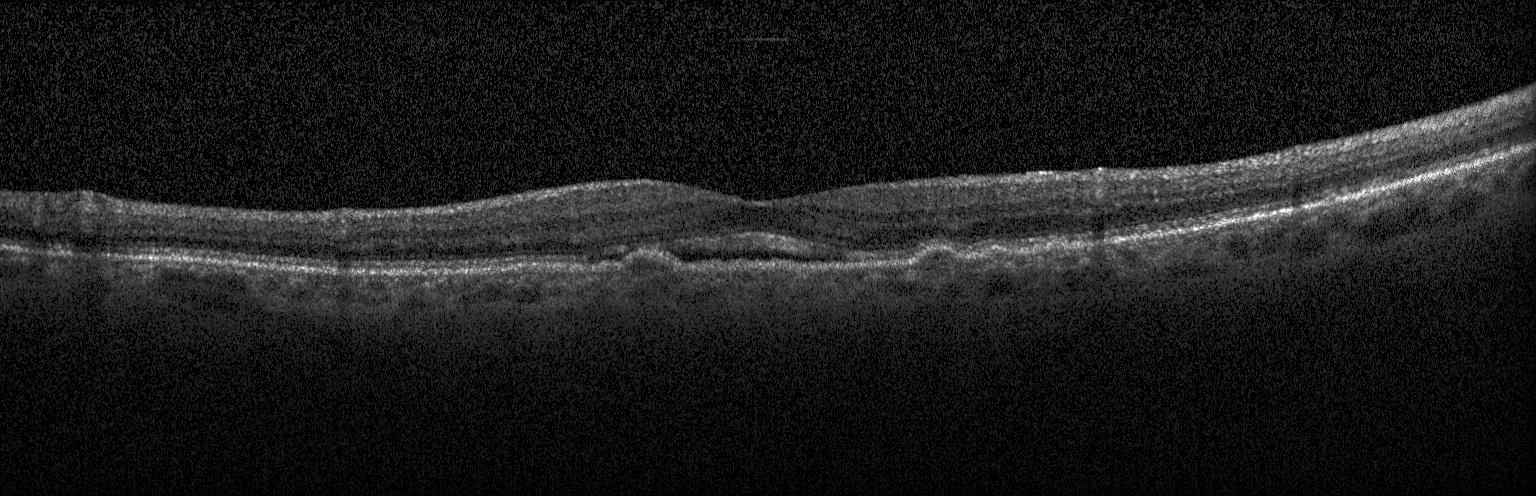

Diagnosis: CNV.